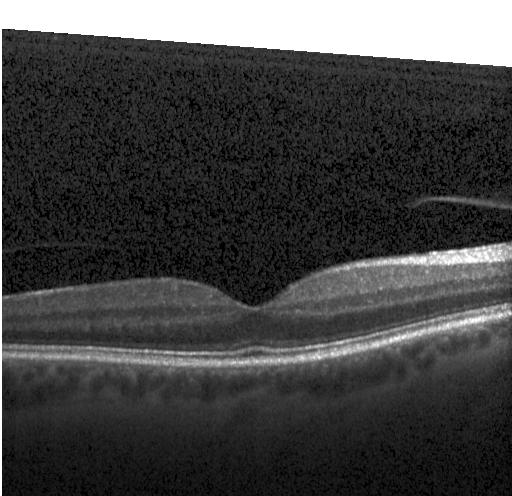

Instrument: Heidelberg Spectralis, horizontal scan through the fovea, SD-OCT, OCT B-scan — Impression: no evidence of CNV, DME, or drusen.